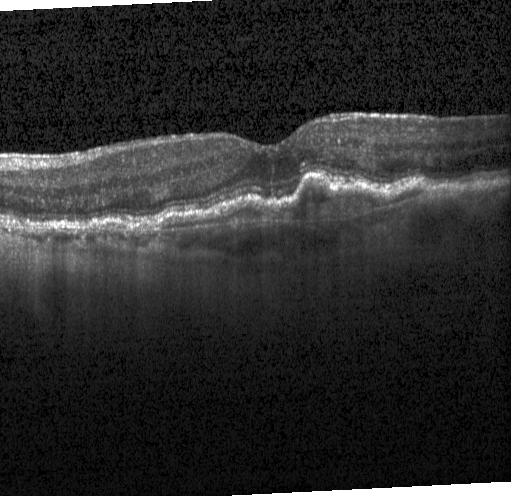
OCT line scan; Heidelberg Spectralis
Finding: choroidal neovascularization.